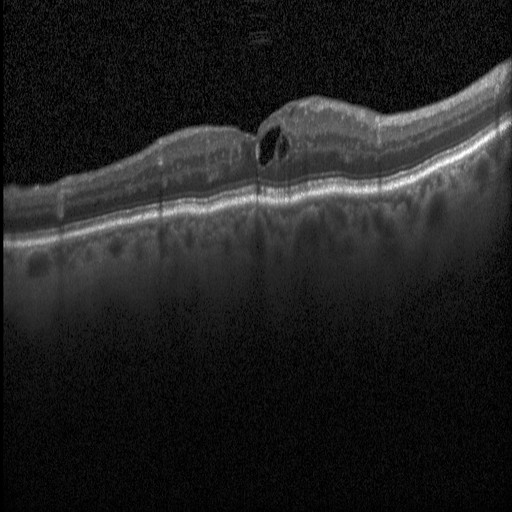 OCT line scan.
This B-scan demonstrates diabetic macular edema (DME).